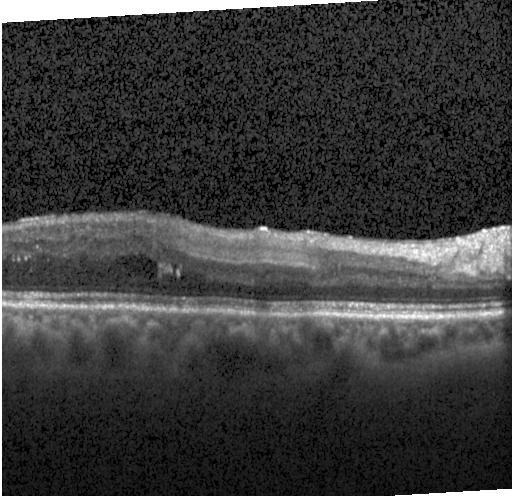
Retinal OCT B-scan — Dx: DME.